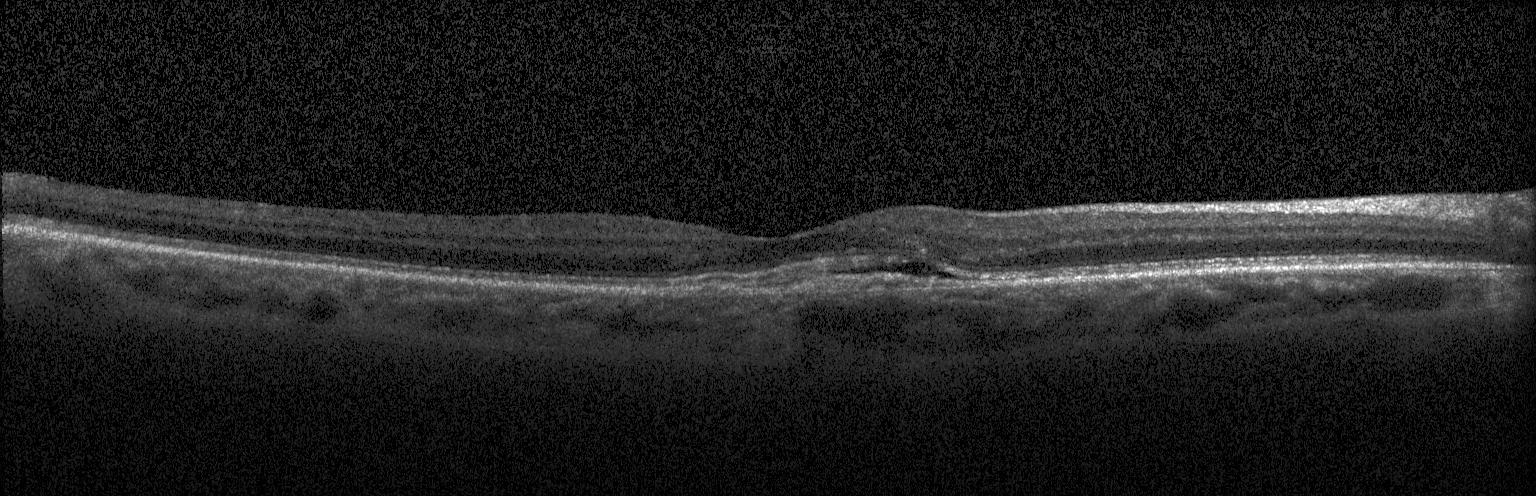
Impression: a choroidal neovascular membrane.